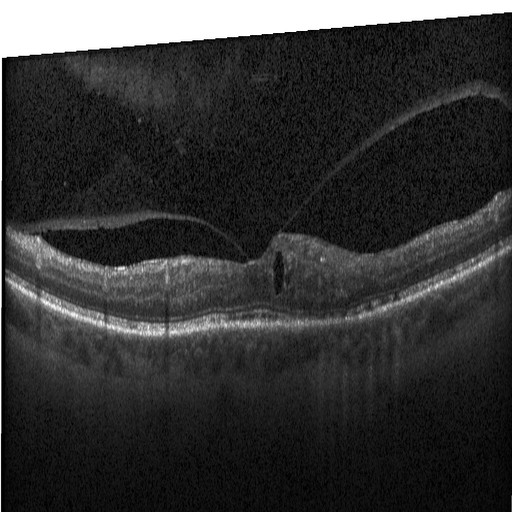 Retinal OCT B-scan — Macular OCT: diabetic macular edema.